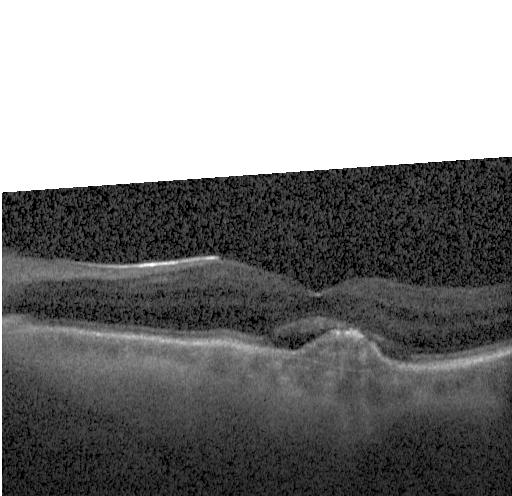
Retinal OCT cross-section showing a choroidal neovascular membrane.